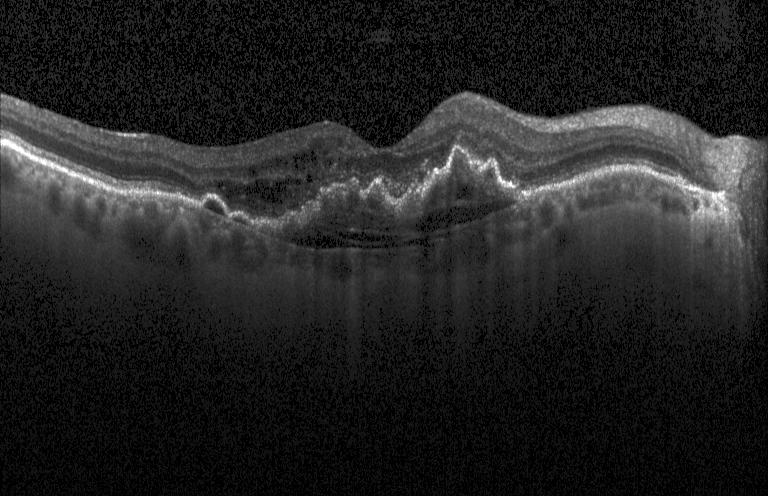 Optical coherence tomography B-scan — Diagnosis: CNV.